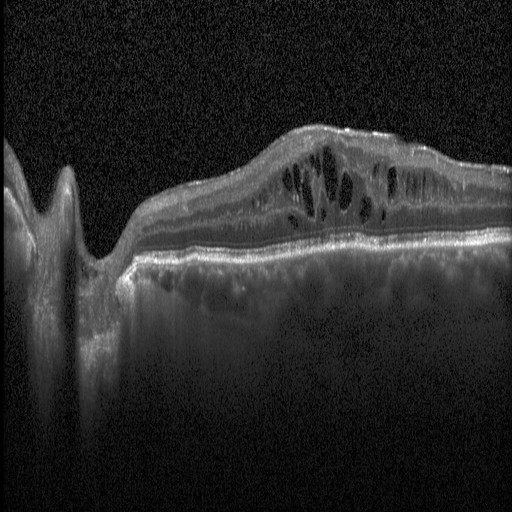
Heidelberg Spectralis. Optical coherence tomography scan. Centered on the fovea. Spectral-domain OCT
Dx: diabetic macular edema (DME).